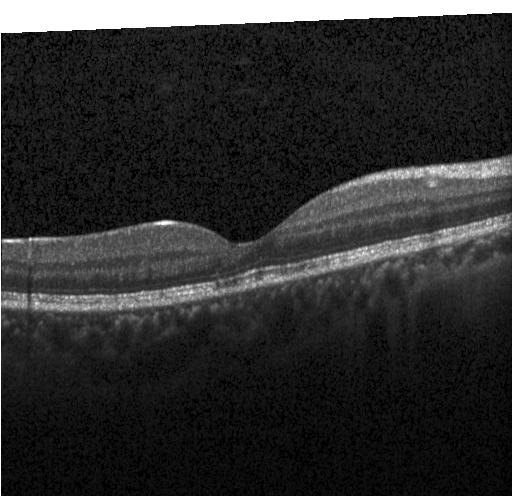
Heidelberg Spectralis OCT system · fovea-centered · OCT B-scan. The scan shows no evidence of choroidal neovascularization, diabetic macular edema, or drusen.